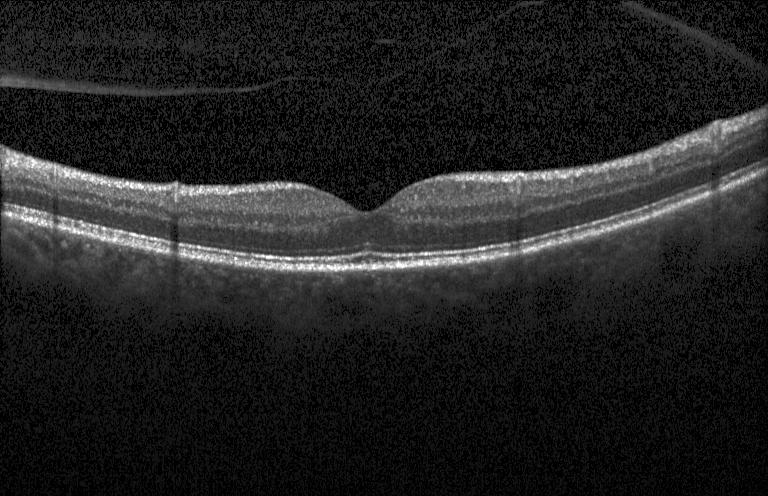
OCT line scan — Impression: no evidence of choroidal neovascularization, diabetic macular edema, or drusen.